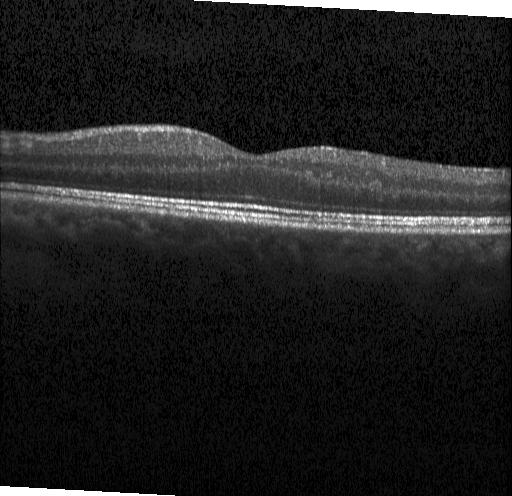 Assessment: no evidence of CNV, DME, or drusen.